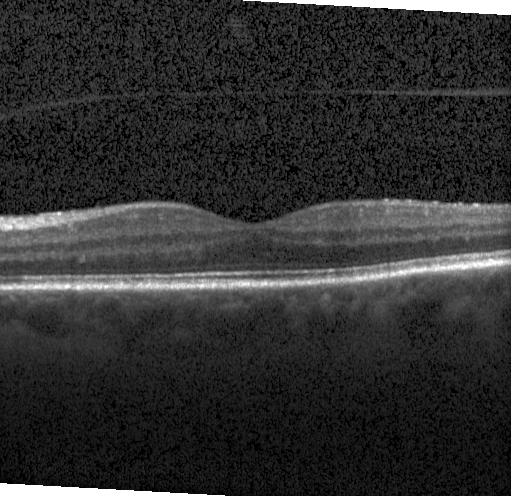
Retinal OCT B-scan, acquired on a Heidelberg Spectralis, horizontal scan through the fovea — No evidence of CNV, DME, or drusen.